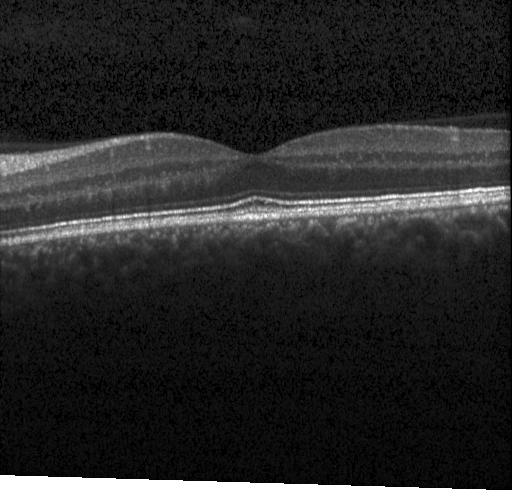 The scan shows no CNV, DME, or drusen.